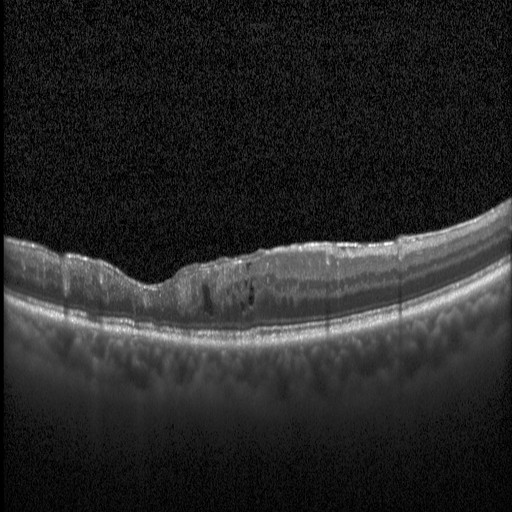
Centered on the fovea, optical coherence tomography B-scan. Diabetic macular edema.